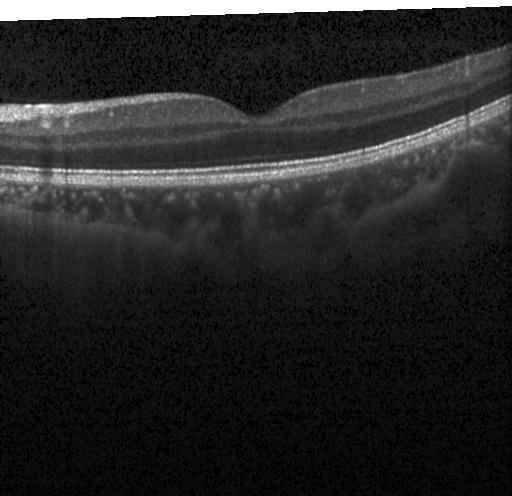 OCT B-scan; Heidelberg Spectralis; fovea-centered. Assessment: no choroidal neovascularization, no diabetic macular edema, and no drusen.